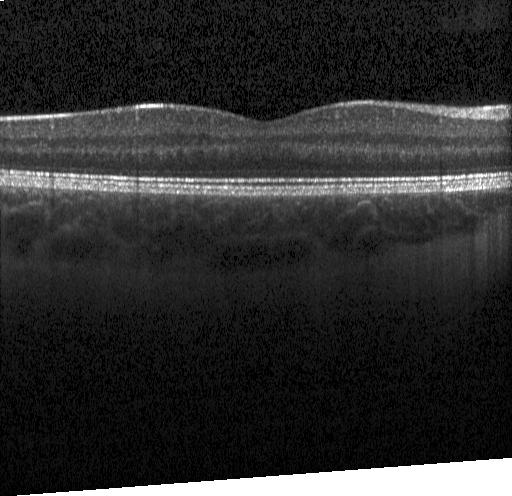

Heidelberg Spectralis OCT system · fovea-centered · optical coherence tomography B-scan. No evidence of choroidal neovascularization, diabetic macular edema, or drusen.